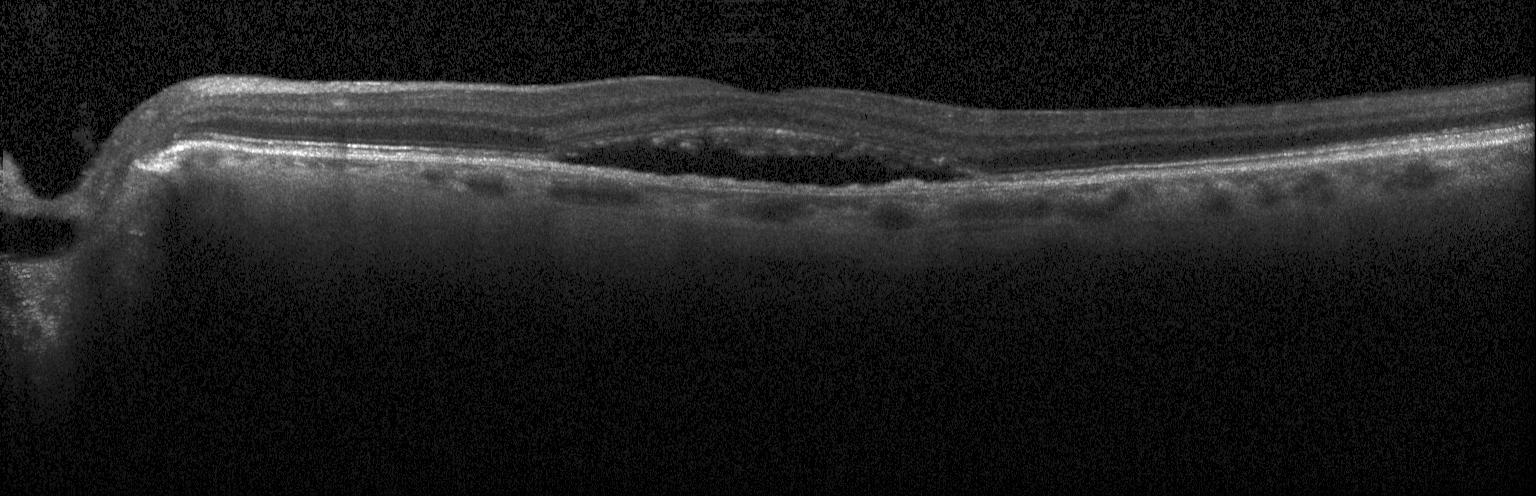 Retinal OCT cross-section, spectral-domain OCT, centered on the fovea, instrument: Heidelberg Spectralis.
Choroidal neovascularization (CNV).